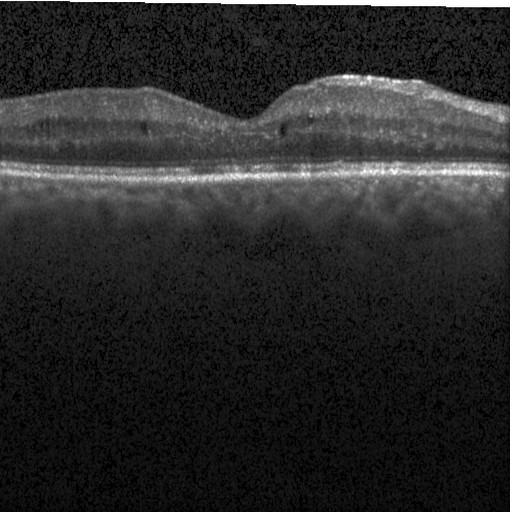
SD-OCT; OCT B-scan; acquired on a Heidelberg Spectralis; macular scan. This B-scan demonstrates diabetic macular edema (DME).